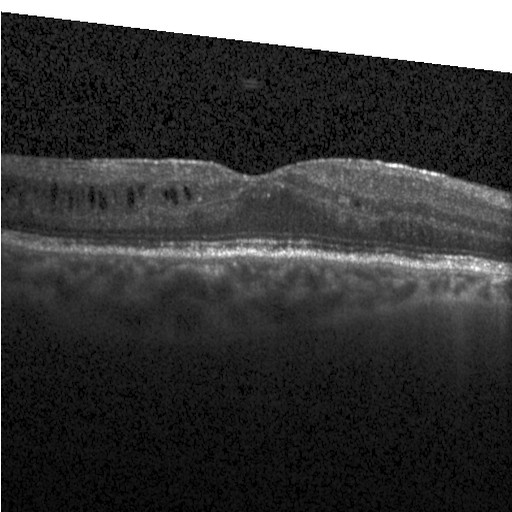

Acquired on a Heidelberg Spectralis; OCT B-scan — OCT finding: DME.